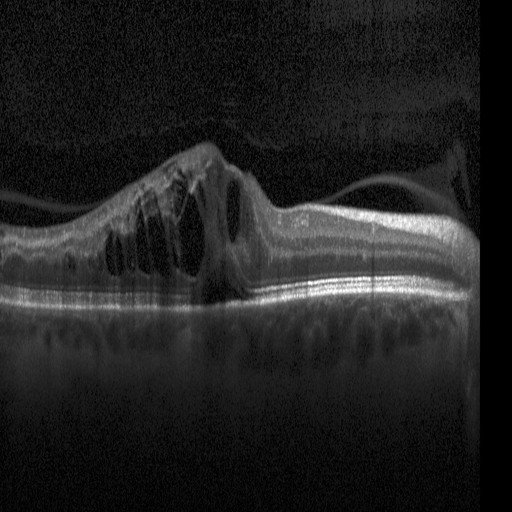
Retinal OCT cross-section showing diabetic macular edema (DME).